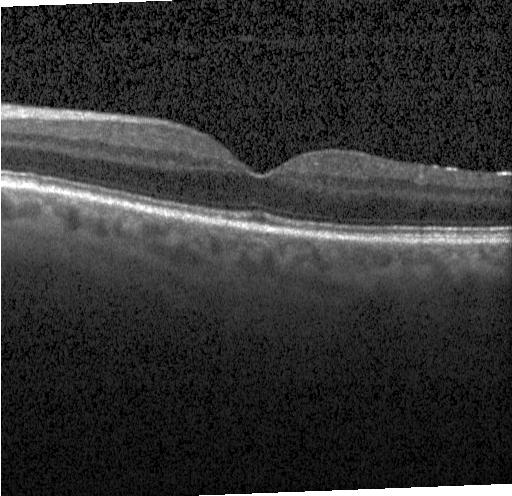

Neither choroidal neovascularization, diabetic macular edema, nor drusen.